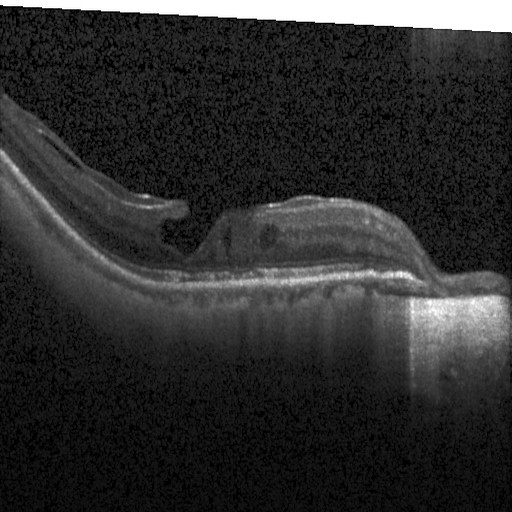
Impression: diabetic macular edema.